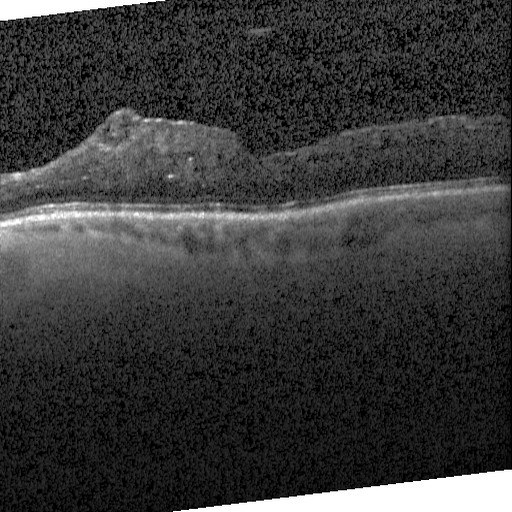
Spectral-domain OCT · optical coherence tomography B-scan
The scan shows diabetic macular edema (DME).